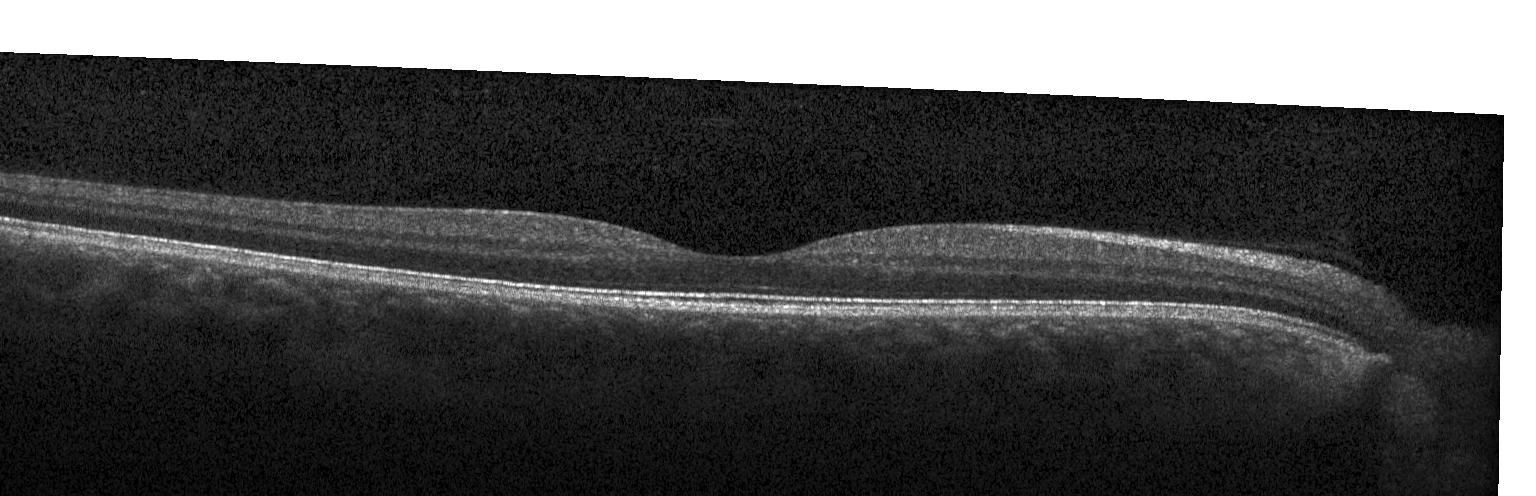
SD-OCT. Macular scan. Retinal OCT cross-section. Heidelberg Spectralis OCT system — Dx: no evidence of CNV, DME, or drusen.